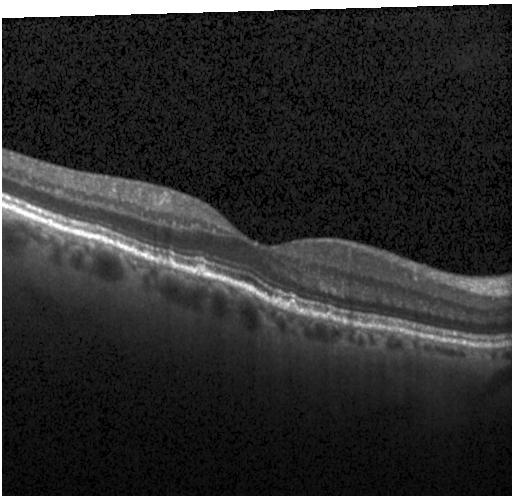

OCT B-scan — Multiple drusen.